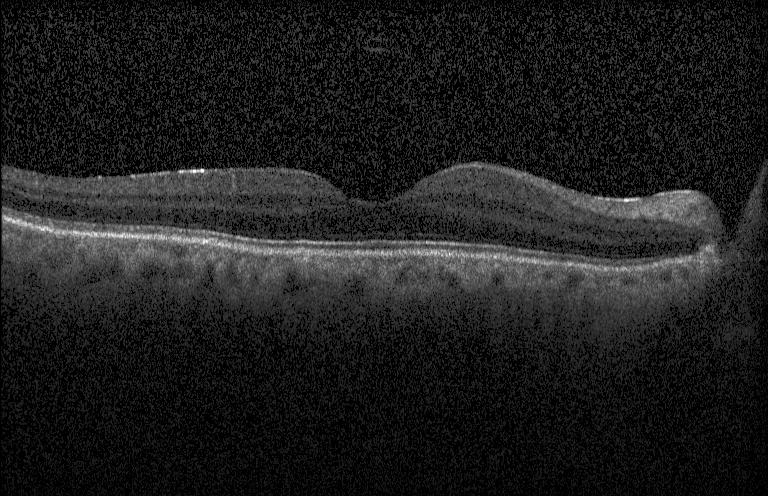 Optical coherence tomography B-scan. Heidelberg Spectralis OCT system. Centered on the fovea. OCT finding: no choroidal neovascularization, diabetic macular edema, or drusen.